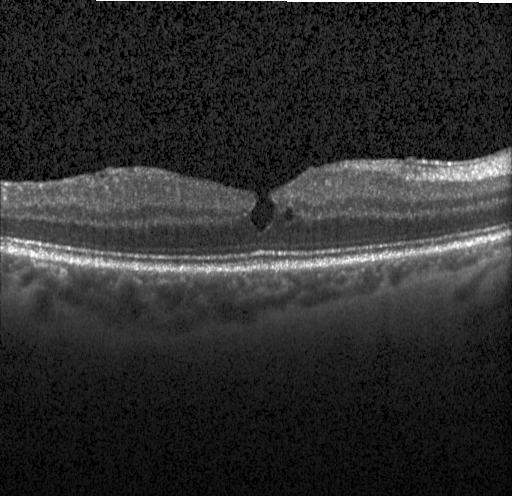

OCT finding: diabetic macular edema.